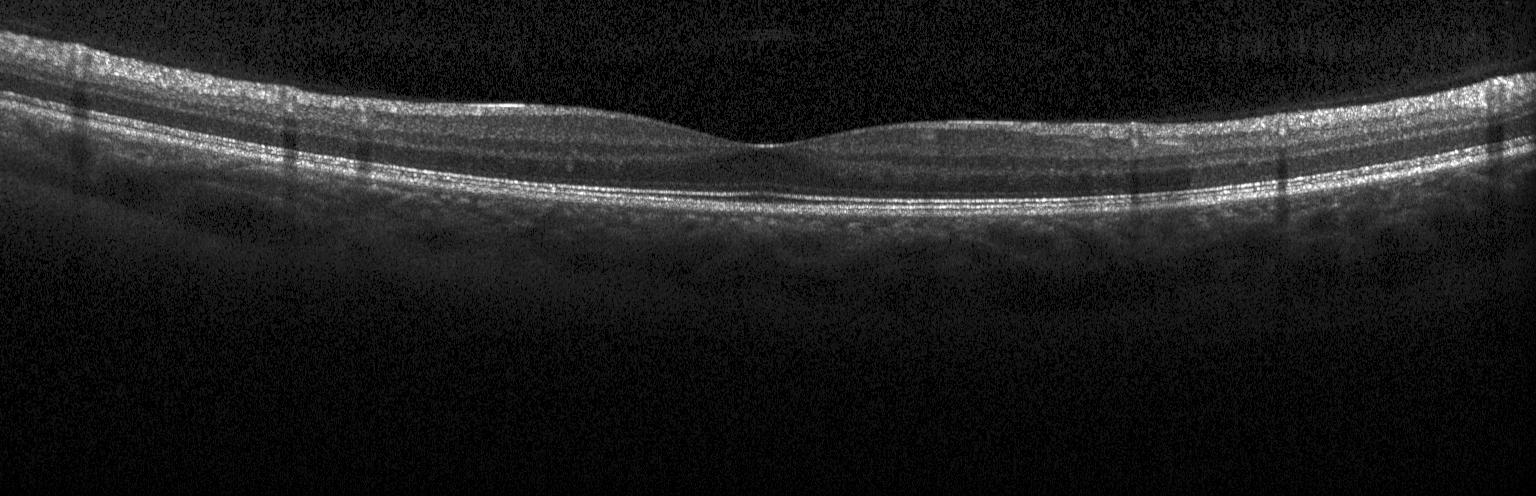 OCT finding: no choroidal neovascularization, diabetic macular edema, or drusen.